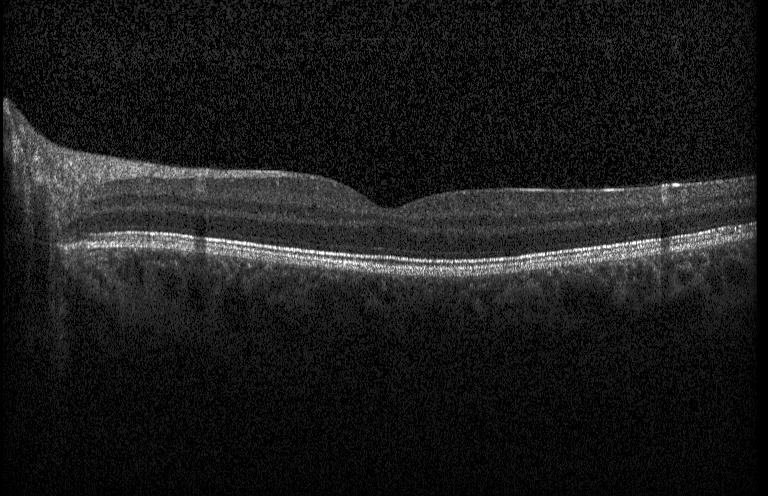
Diagnosis: no evidence of CNV, DME, or drusen.